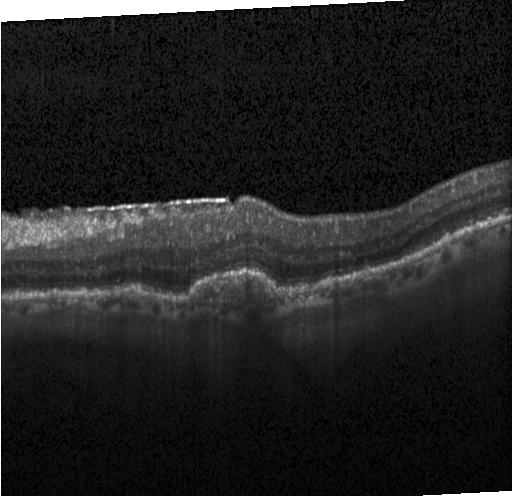 Optical coherence tomography scan. Finding: a choroidal neovascular membrane.